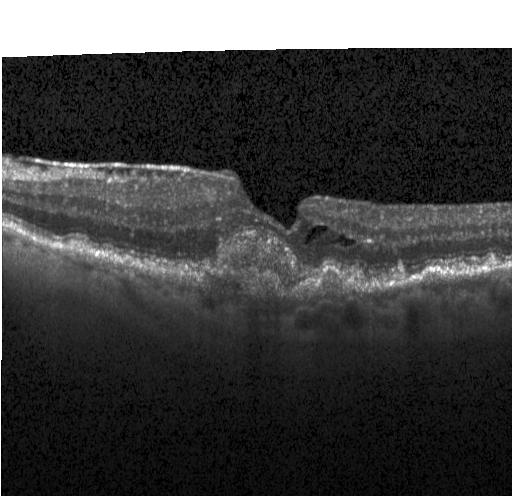
Retinal OCT cross-section; horizontal scan through the fovea; Heidelberg Spectralis OCT system; spectral-domain optical coherence tomography
Diagnosis: CNV.